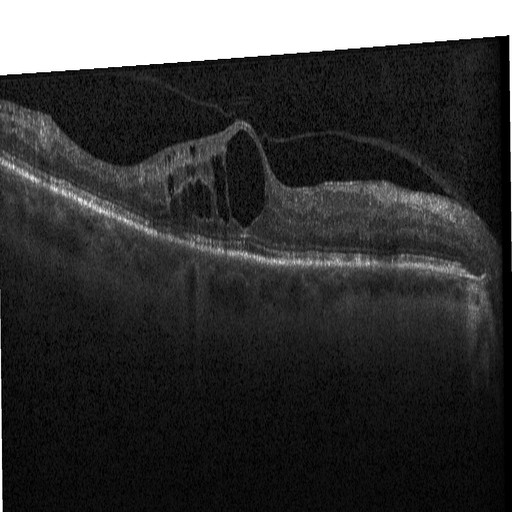
OCT finding: DME.